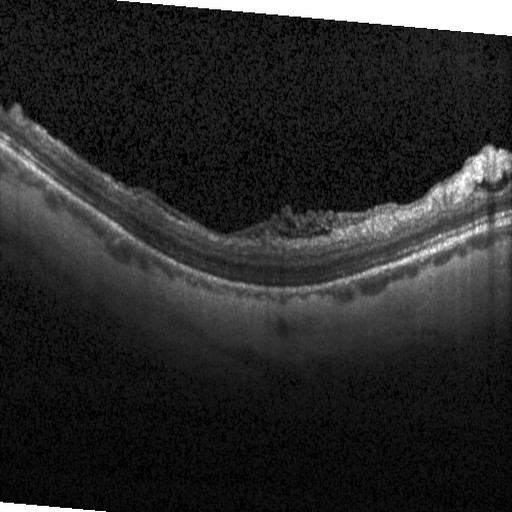

Heidelberg Spectralis, OCT line scan
Diagnosis: diabetic macular edema.